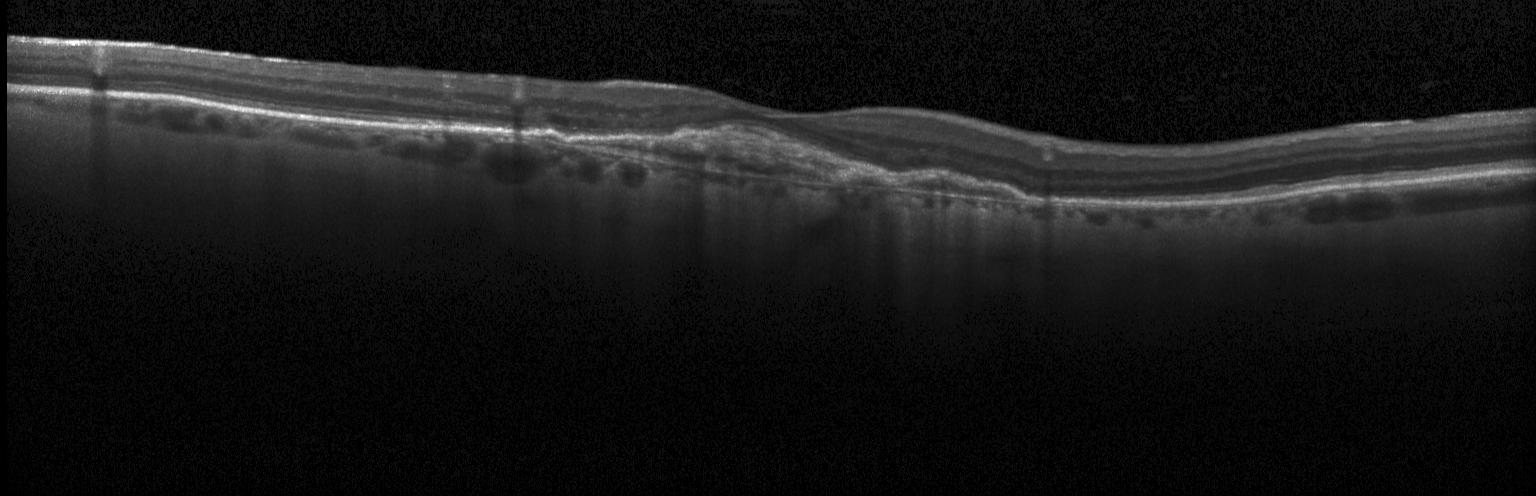
OCT B-scan showing CNV.